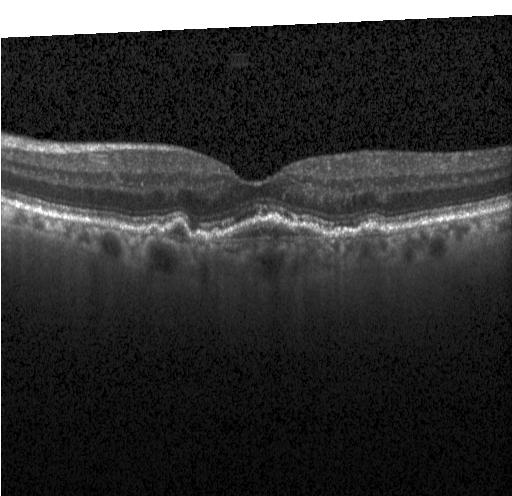
OCT finding: a choroidal neovascular membrane.